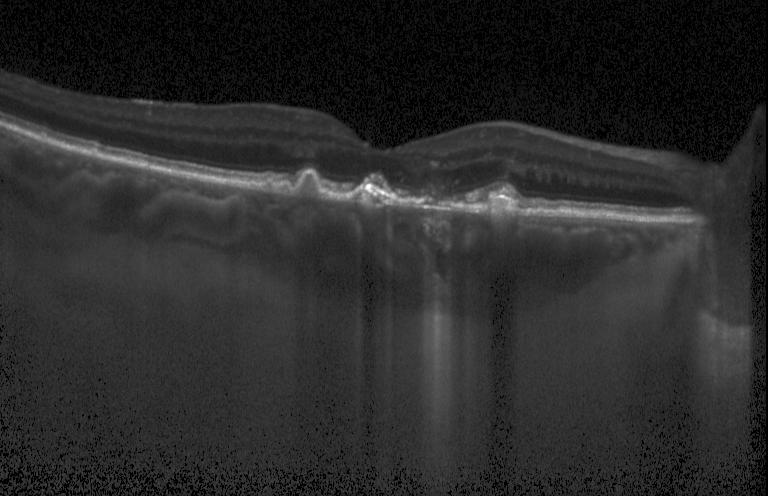 Retinal OCT cross-section — Finding: a choroidal neovascular membrane.